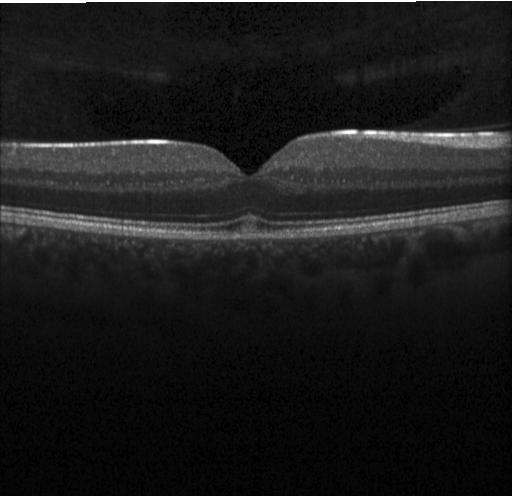

Fovea-centered. Acquired on a Heidelberg Spectralis. Retinal OCT cross-section. Spectral-domain optical coherence tomography — Finding: neither choroidal neovascularization, diabetic macular edema, nor drusen.